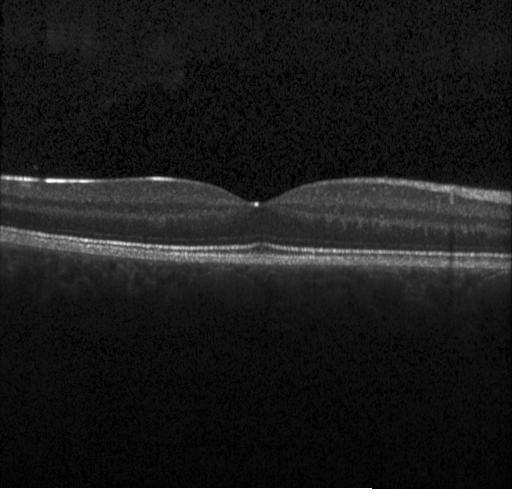 OCT B-scan.
Macular OCT: no choroidal neovascularization, no diabetic macular edema, and no drusen.